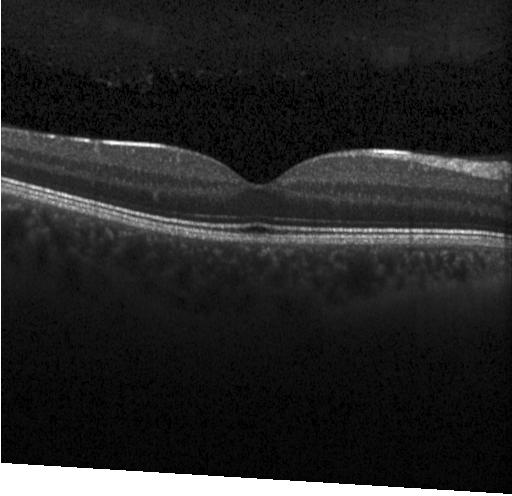
Spectral-domain OCT B-scan: no choroidal neovascularization, no diabetic macular edema, and no drusen.